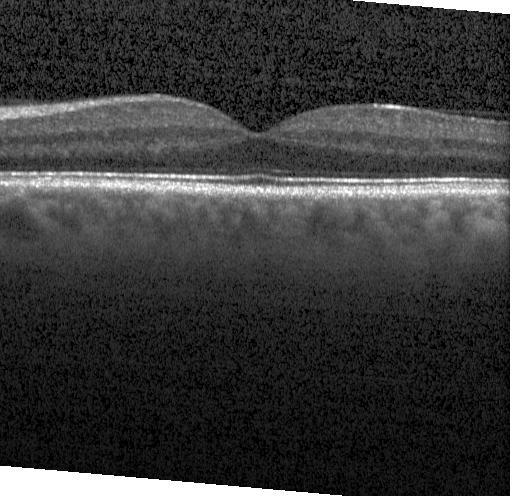
SD-OCT. Retinal OCT cross-section. Heidelberg Spectralis.
Dx: neither choroidal neovascularization, diabetic macular edema, nor drusen.